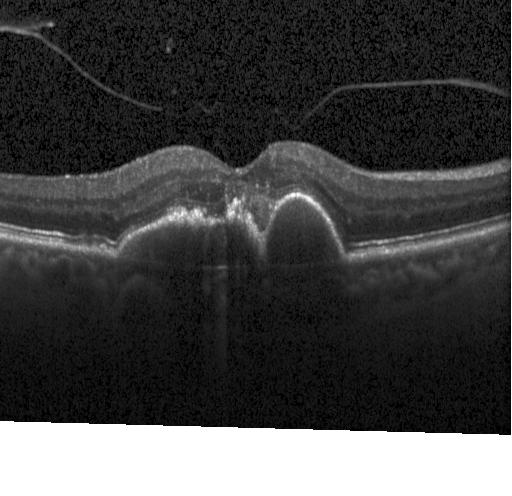
Optical coherence tomography scan — Macular OCT: a choroidal neovascular membrane.